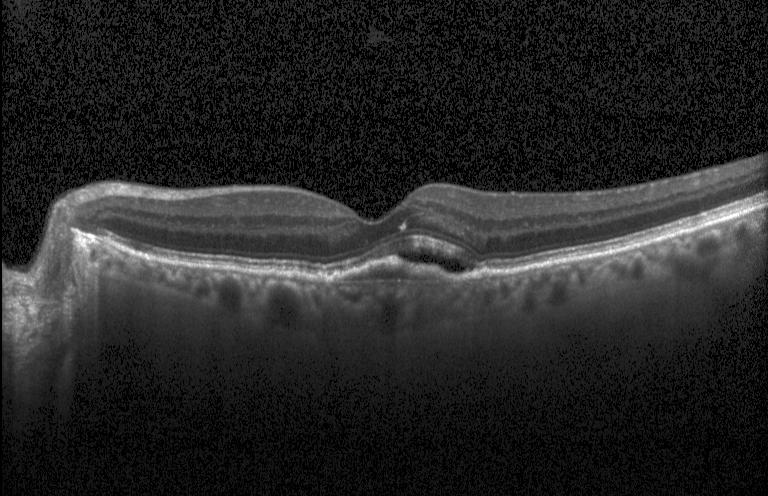

Retinal OCT cross-section.
Impression: choroidal neovascularization.